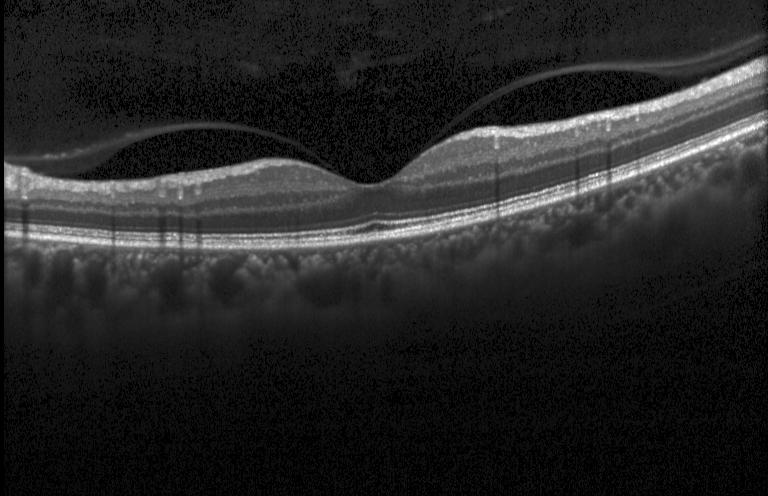
Retinal OCT cross-section · horizontal scan through the fovea · spectral-domain optical coherence tomography · Heidelberg Spectralis. OCT finding: no CNV, no DME, and no drusen.